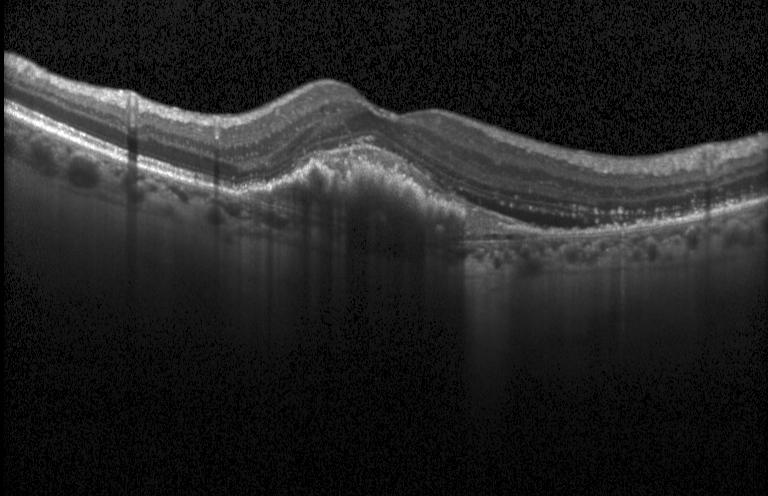 Dx: a choroidal neovascular membrane.